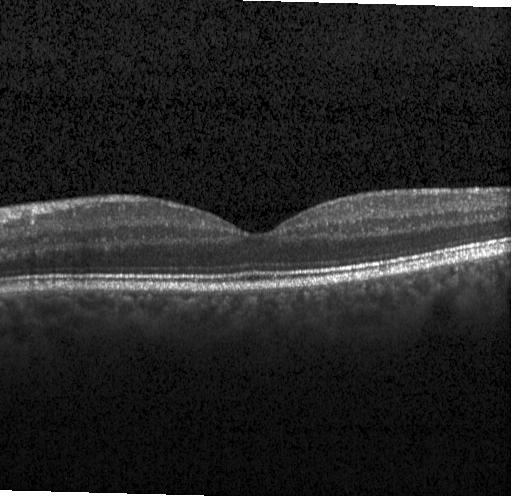 OCT scan showing no evidence of CNV, DME, or drusen.